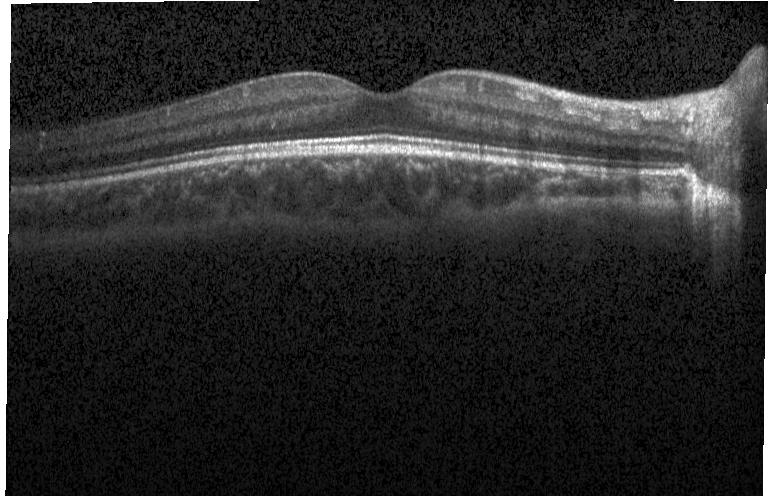

SD-OCT. Retinal OCT B-scan.
No CNV, DME, or drusen.